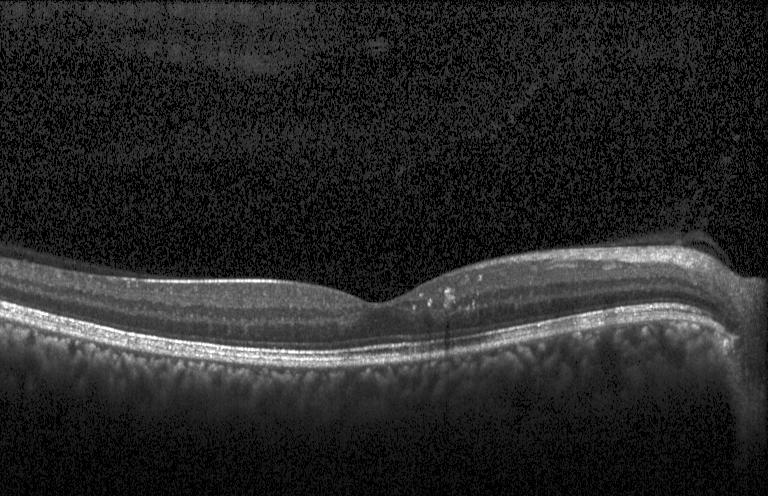
Retinal OCT cross-section.
Macular OCT: neither choroidal neovascularization, diabetic macular edema, nor drusen.